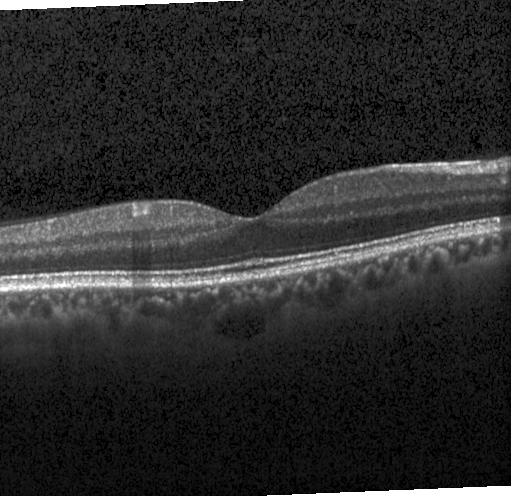
OCT line scan; macular scan
Diagnosis: no evidence of CNV, DME, or drusen.